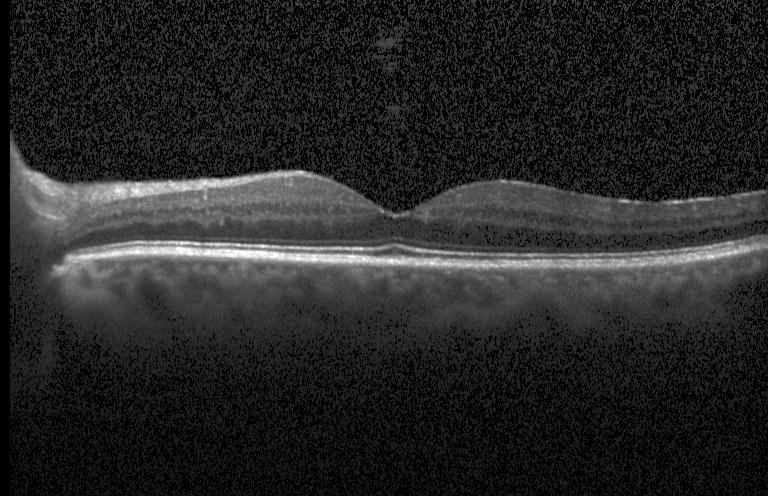

Heidelberg Spectralis. Centered on the fovea. Optical coherence tomography B-scan
The scan shows neither choroidal neovascularization, diabetic macular edema, nor drusen.